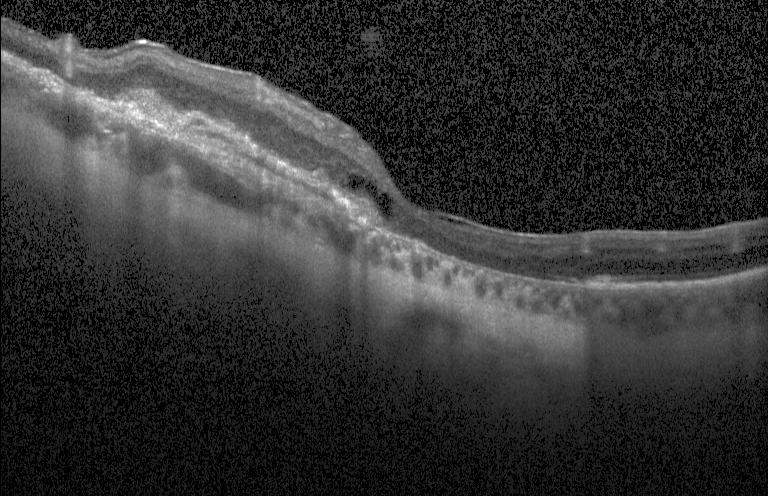

The scan shows CNV.